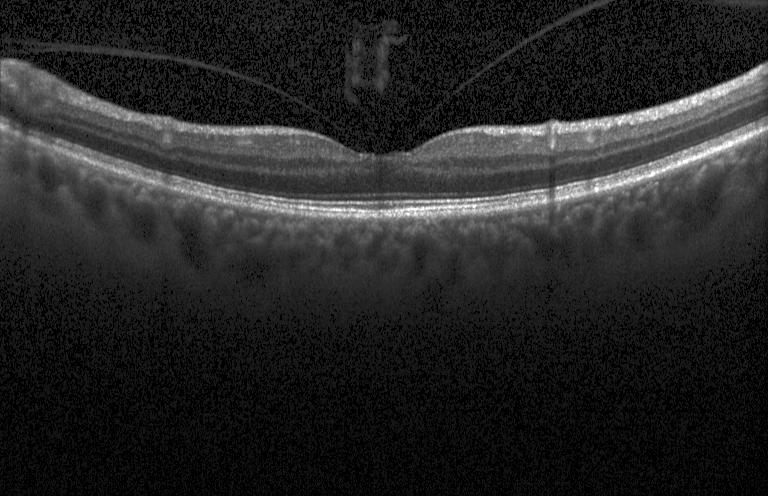
Spectral-domain OCT B-scan: no evidence of choroidal neovascularization, diabetic macular edema, or drusen.